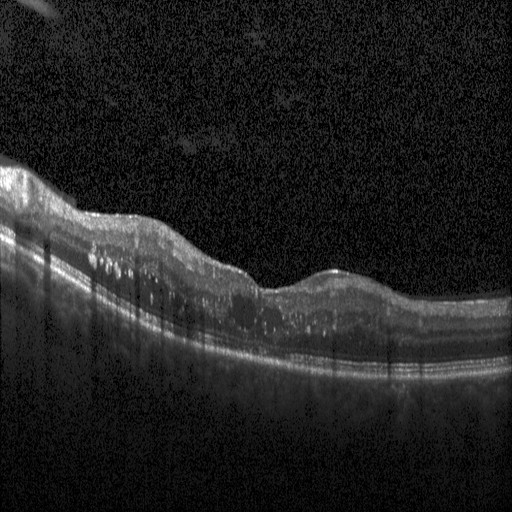

OCT B-scan, macular scan — Diagnosis: diabetic macular edema (DME).